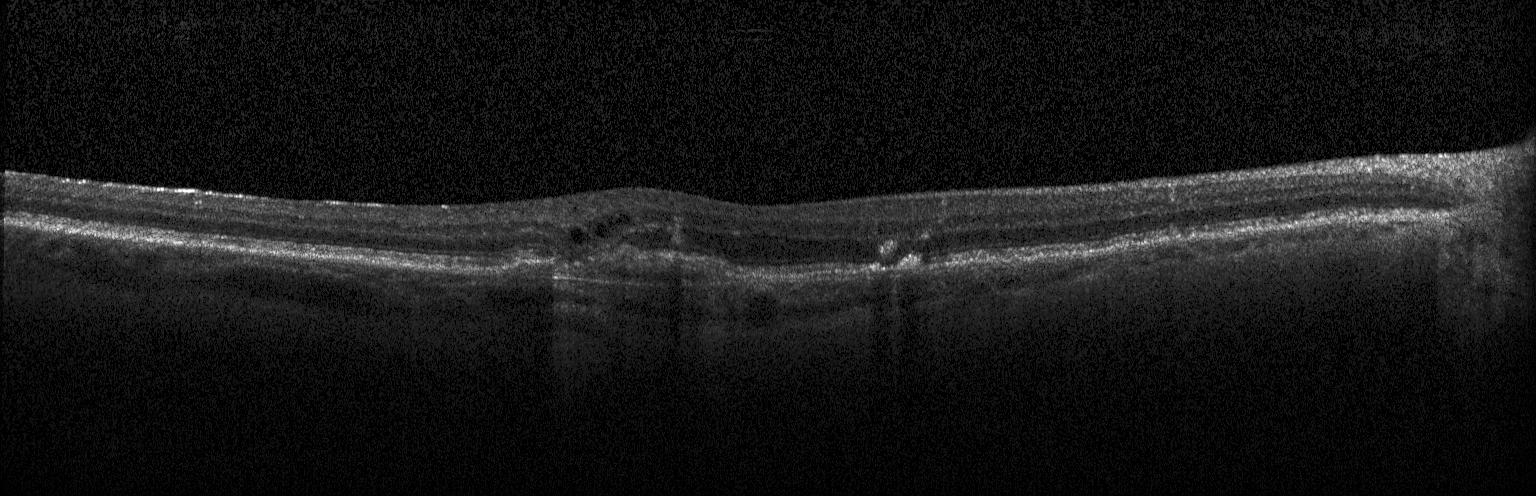 Optical coherence tomography scan.
Assessment: a choroidal neovascular membrane.